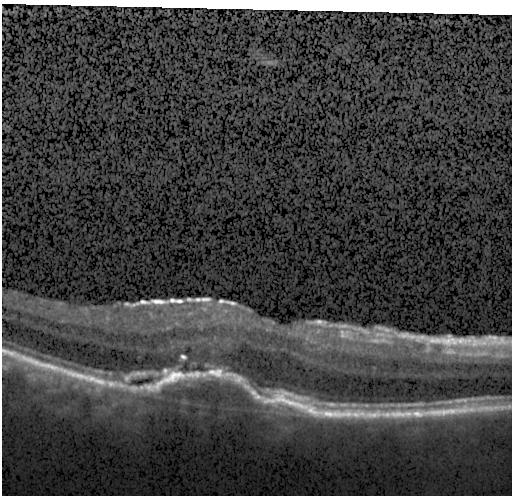
OCT scan showing a choroidal neovascular membrane.